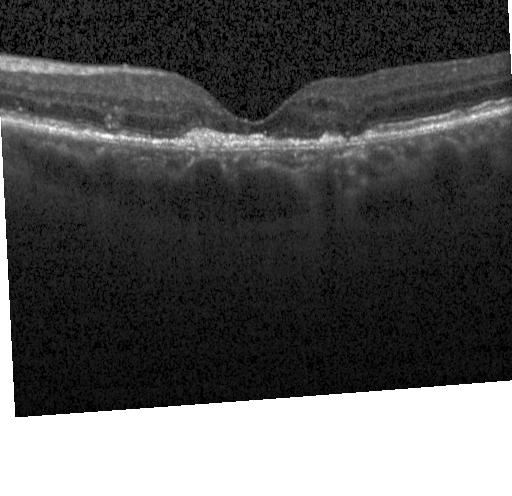 Heidelberg Spectralis OCT system; optical coherence tomography scan. Impression: choroidal neovascularization.